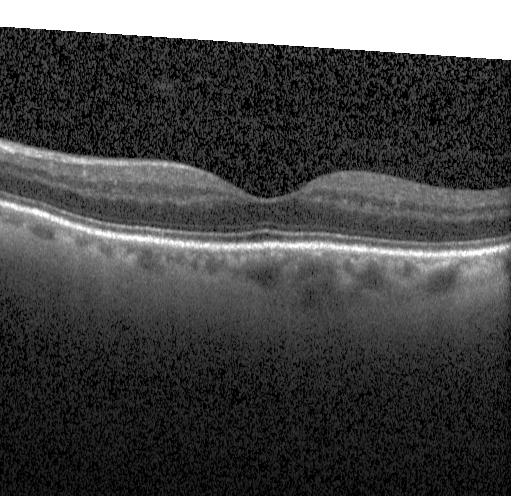
Optical coherence tomography scan. Impression: no evidence of choroidal neovascularization, diabetic macular edema, or drusen.